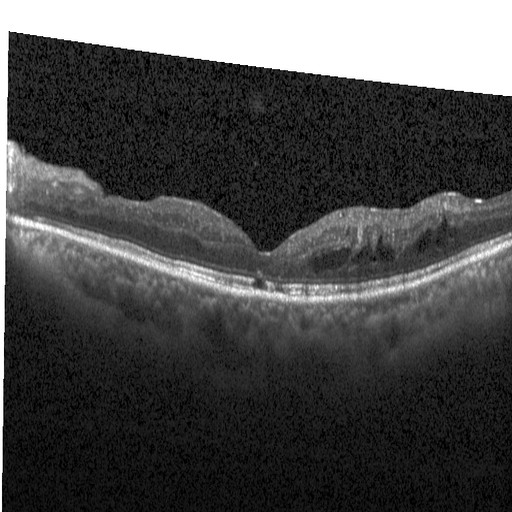 Heidelberg Spectralis. OCT B-scan. Macular scan. Spectral-domain optical coherence tomography. Diagnosis: DME.